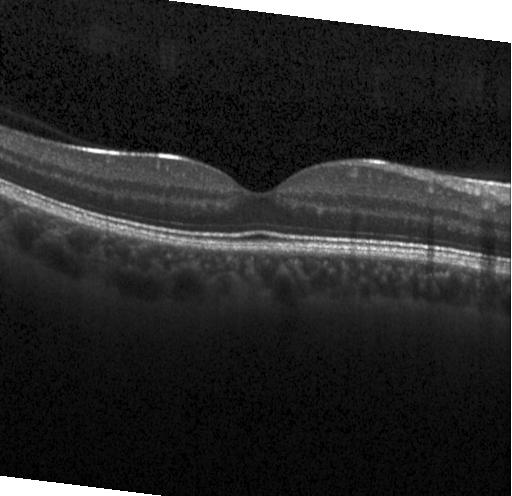
Retinal OCT cross-section
This B-scan demonstrates no evidence of choroidal neovascularization, diabetic macular edema, or drusen.